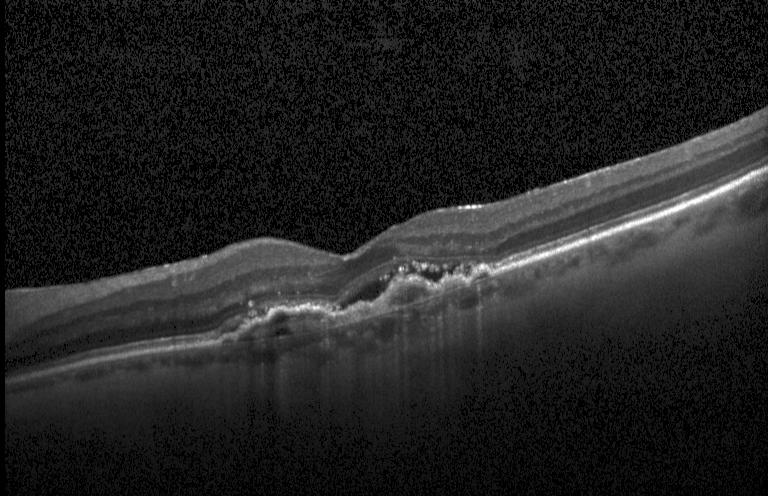

OCT line scan
Diagnosis: a choroidal neovascular membrane.